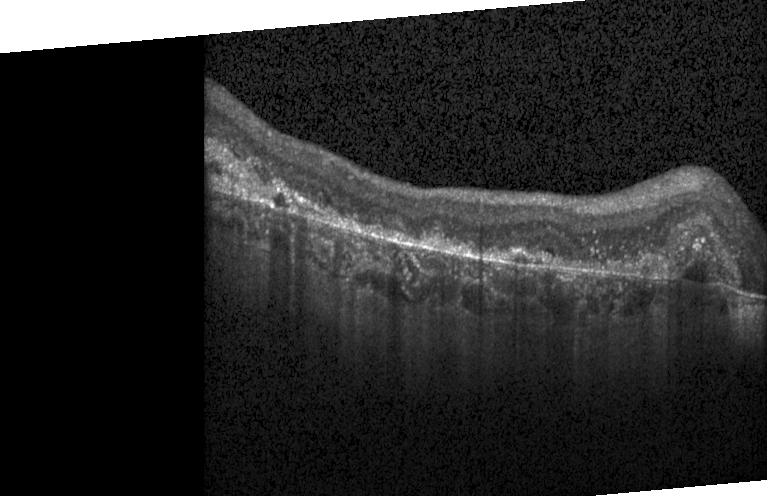
Impression: a choroidal neovascular membrane.